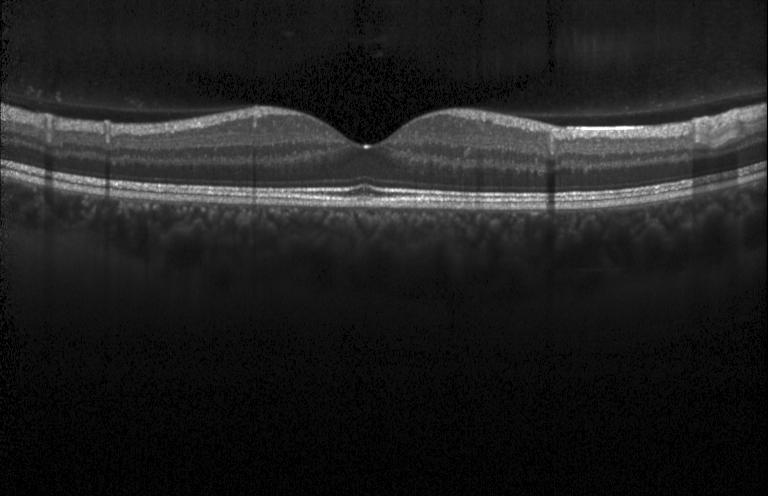 Diagnosis: no evidence of CNV, DME, or drusen.